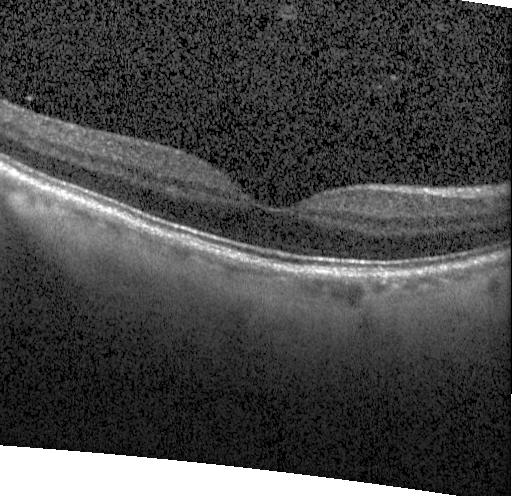 Optical coherence tomography B-scan. Finding: no evidence of choroidal neovascularization, diabetic macular edema, or drusen.